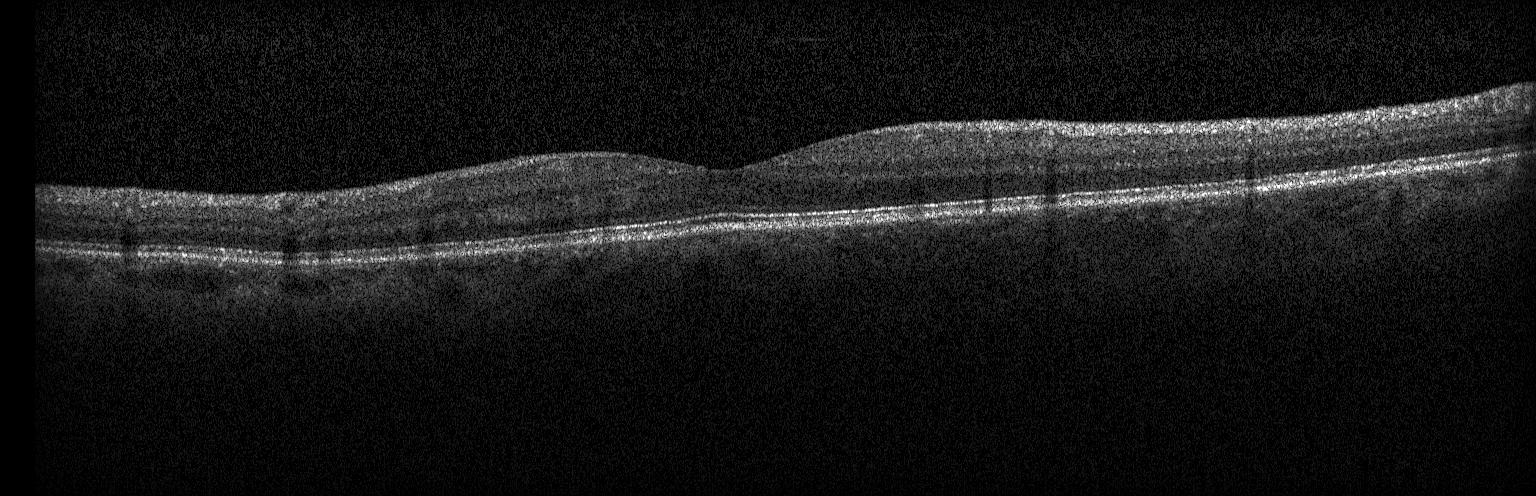
Heidelberg Spectralis OCT system. Spectral-domain OCT. OCT line scan
Diagnosis: no evidence of choroidal neovascularization, diabetic macular edema, or drusen.